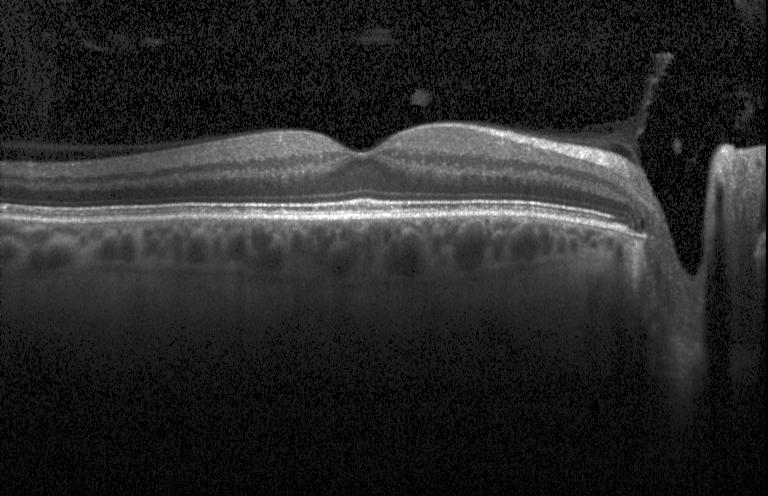

Acquired on a Heidelberg Spectralis, macular scan, OCT line scan, spectral-domain optical coherence tomography — Impression: no evidence of choroidal neovascularization, diabetic macular edema, or drusen.